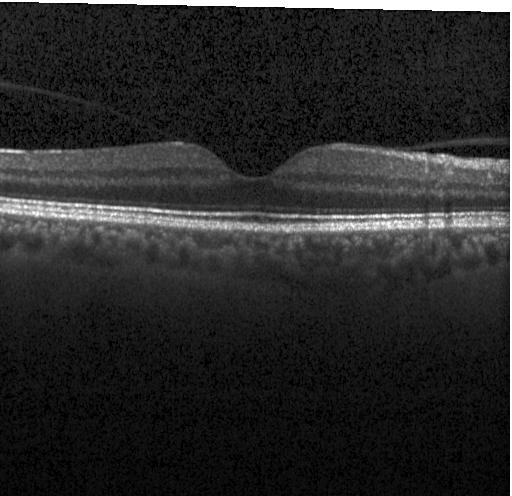

OCT B-scan showing no CNV, DME, or drusen.